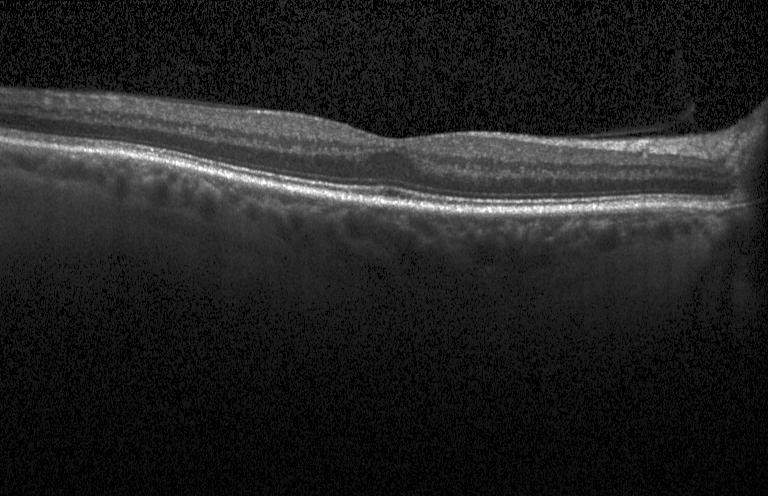 Horizontal scan through the fovea · optical coherence tomography scan
Diagnosis: no evidence of choroidal neovascularization, diabetic macular edema, or drusen.